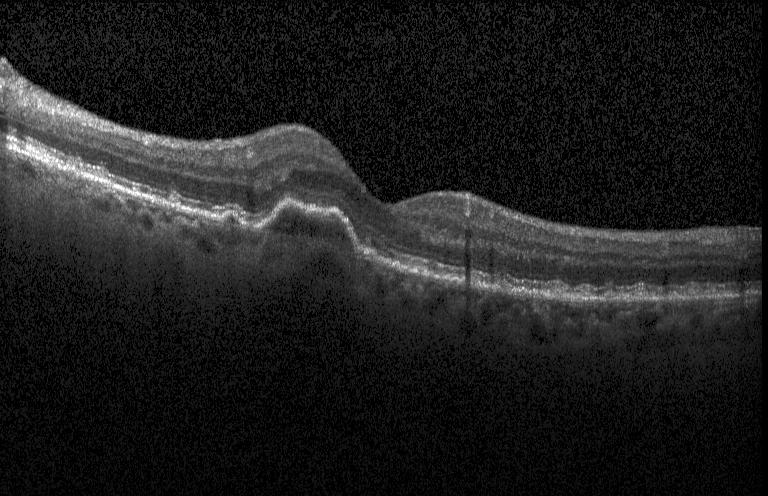 SD-OCT; centered on the fovea; OCT line scan; acquired on a Heidelberg Spectralis. Choroidal neovascularization (CNV).